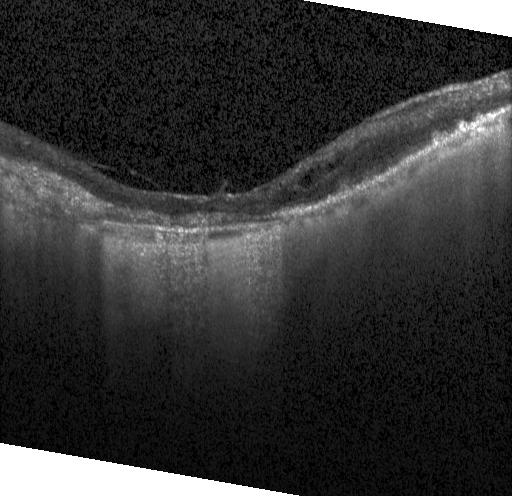
OCT B-scan, Heidelberg Spectralis OCT system, spectral-domain optical coherence tomography — Assessment: a choroidal neovascular membrane.